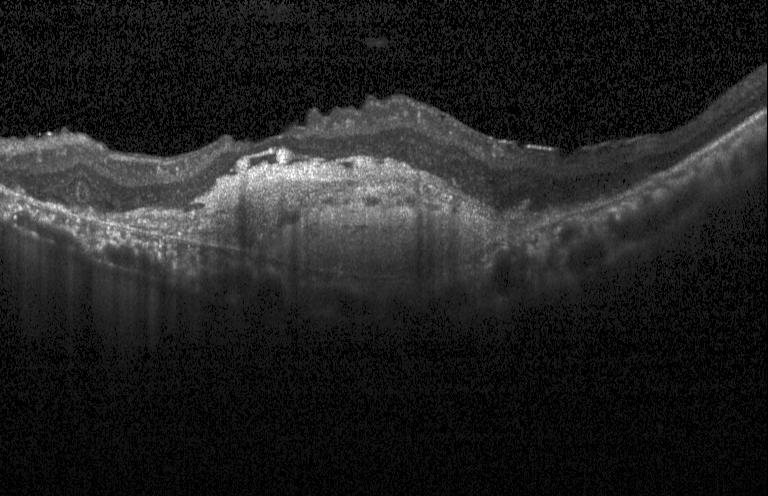

Impression: a choroidal neovascular membrane.